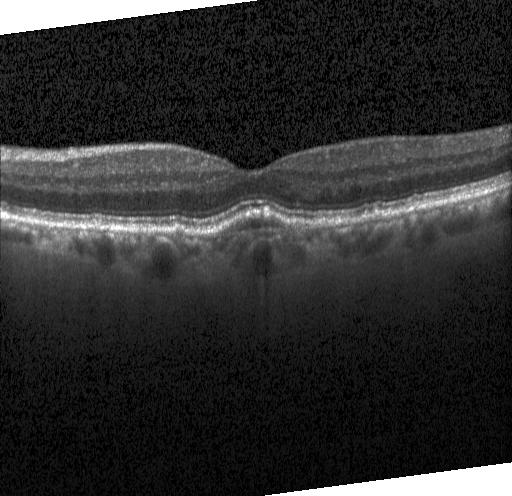

Macular OCT demonstrating choroidal neovascularization (CNV).